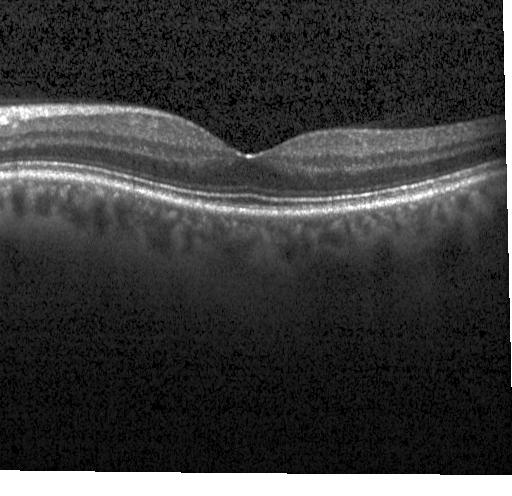

OCT B-scan.
OCT finding: no CNV, no DME, and no drusen.